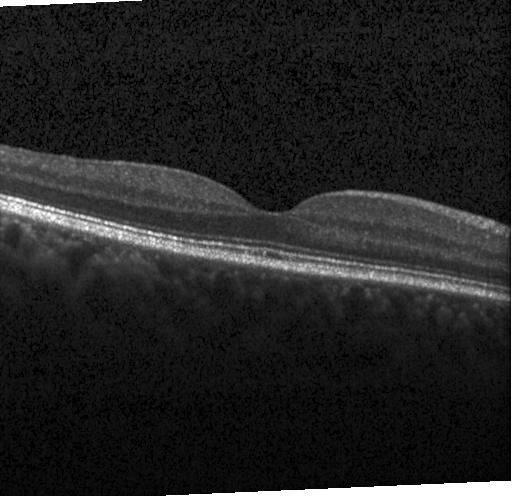
This B-scan demonstrates no evidence of CNV, DME, or drusen.